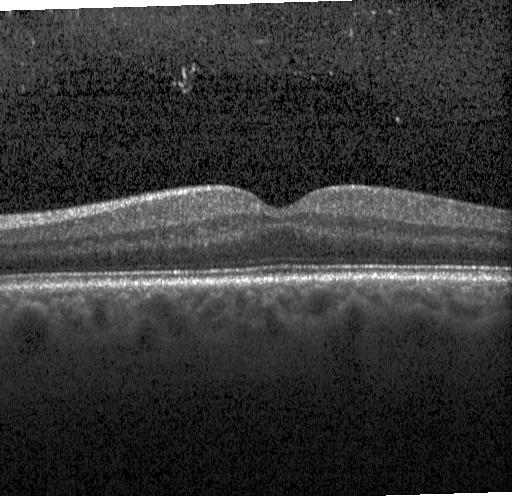 OCT scan showing neither choroidal neovascularization, diabetic macular edema, nor drusen.